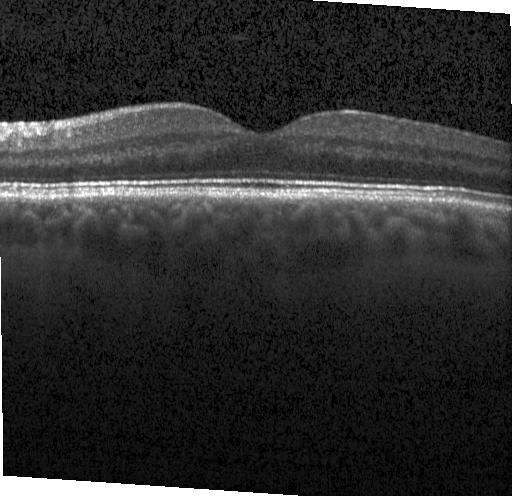 Instrument: Heidelberg Spectralis; centered on the fovea; OCT line scan.
Finding: no CNV, no DME, and no drusen.